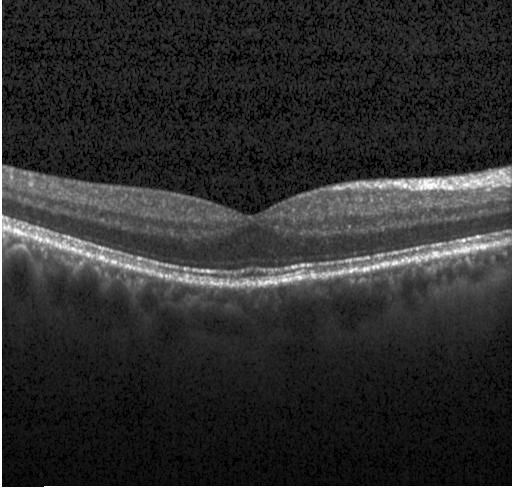
Finding: no choroidal neovascularization, diabetic macular edema, or drusen.